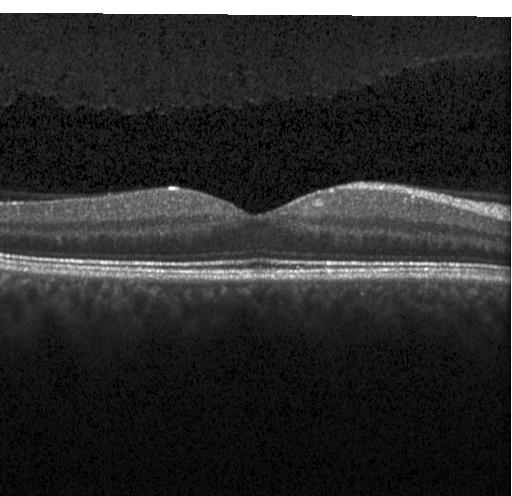 Heidelberg Spectralis OCT system. Optical coherence tomography B-scan. Assessment: no CNV, no DME, and no drusen.